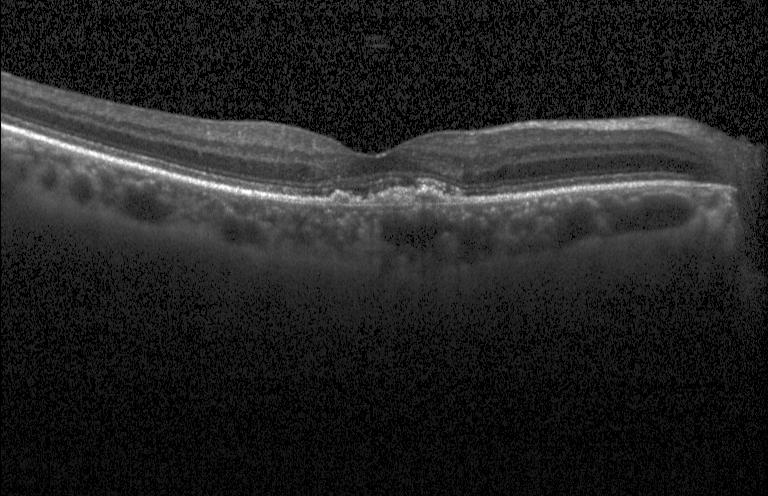

OCT B-scan showing a choroidal neovascular membrane.